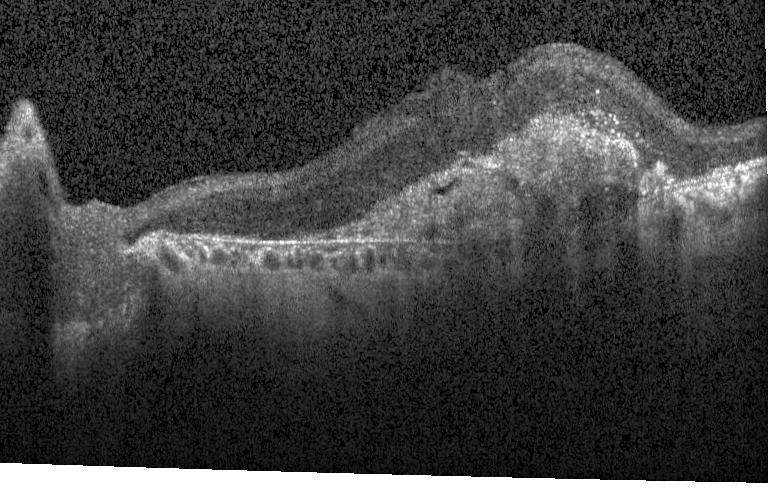
Assessment: a choroidal neovascular membrane.